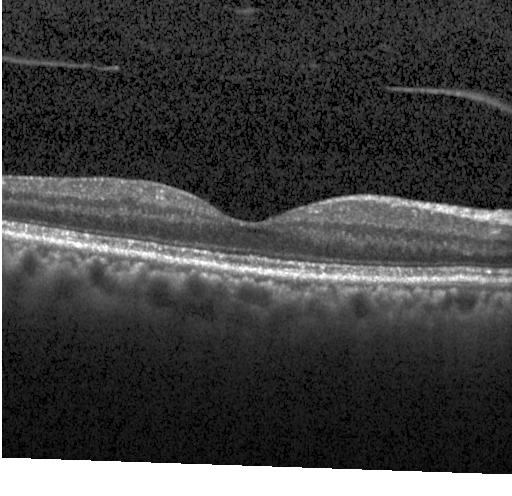 Spectral-domain optical coherence tomography · OCT B-scan · instrument: Heidelberg Spectralis.
Dx: no choroidal neovascularization, no diabetic macular edema, and no drusen.